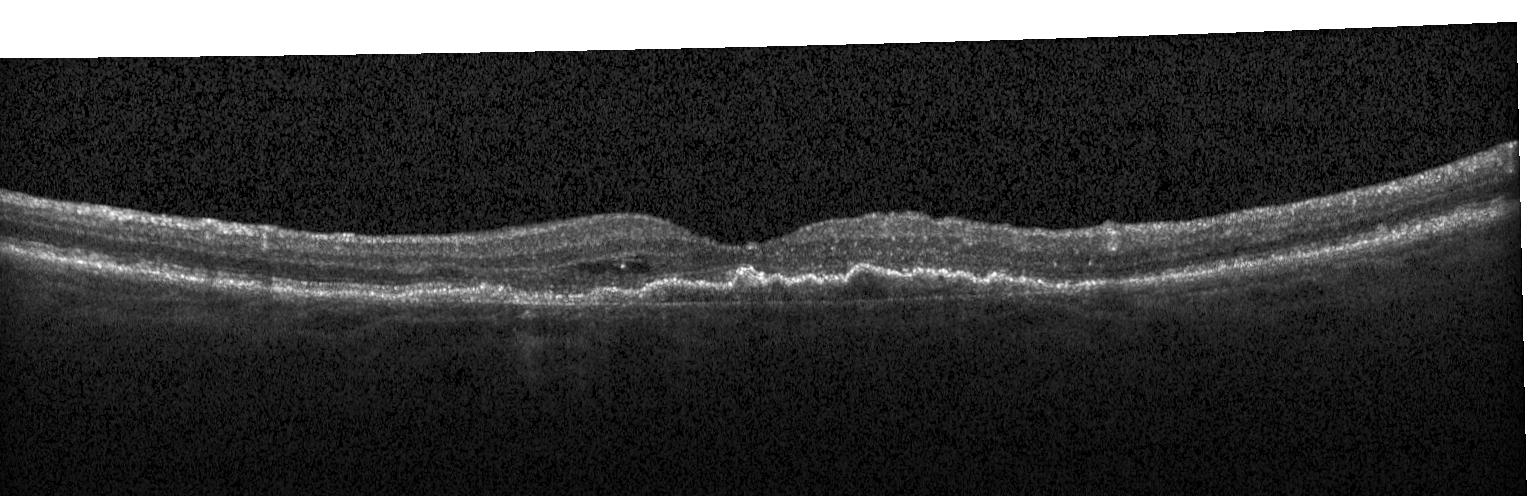

SD-OCT, retinal OCT B-scan, acquired on a Heidelberg Spectralis — This B-scan demonstrates CNV.